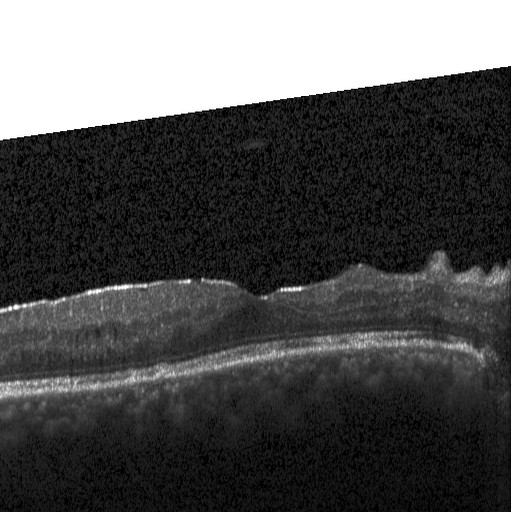
Retinal OCT B-scan.
Impression: diabetic macular edema (DME).